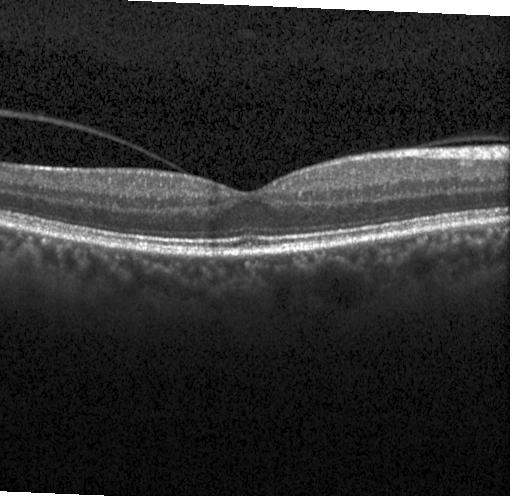

Optical coherence tomography scan · SD-OCT · horizontal scan through the fovea
Finding: no evidence of choroidal neovascularization, diabetic macular edema, or drusen.